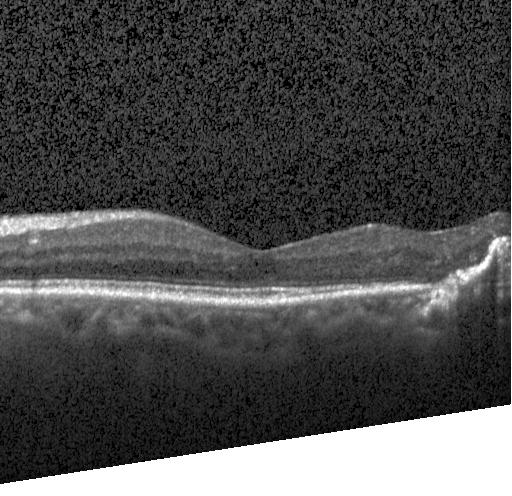 Diagnosis: choroidal neovascularization (CNV).